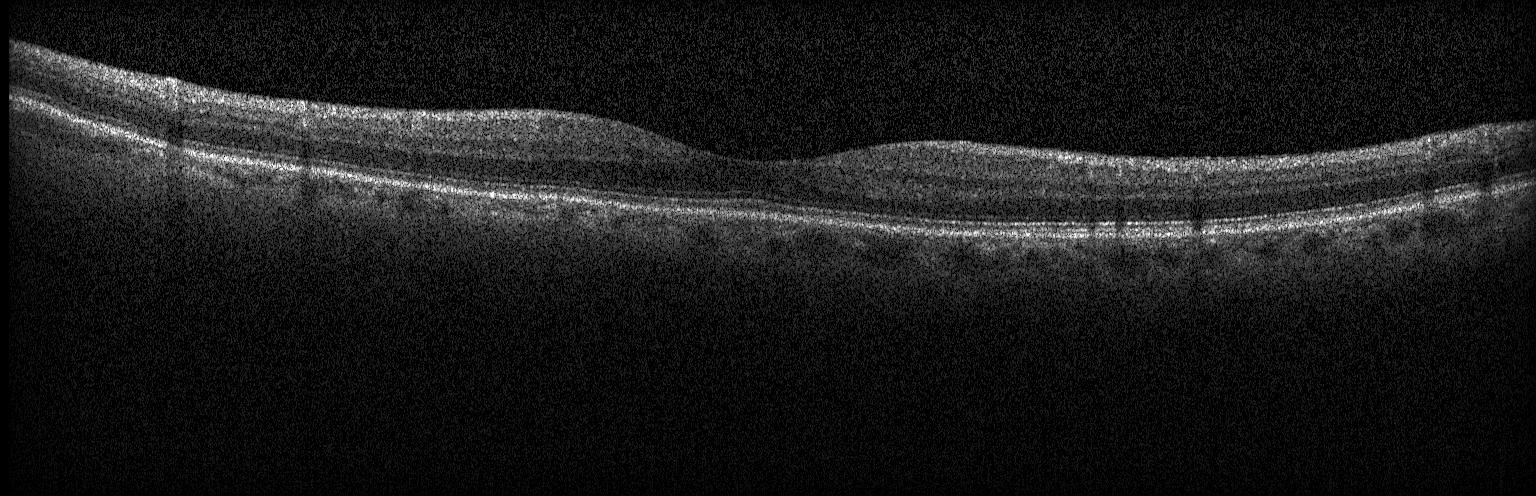
Macular scan; retinal OCT B-scan
Impression: no choroidal neovascularization, diabetic macular edema, or drusen.